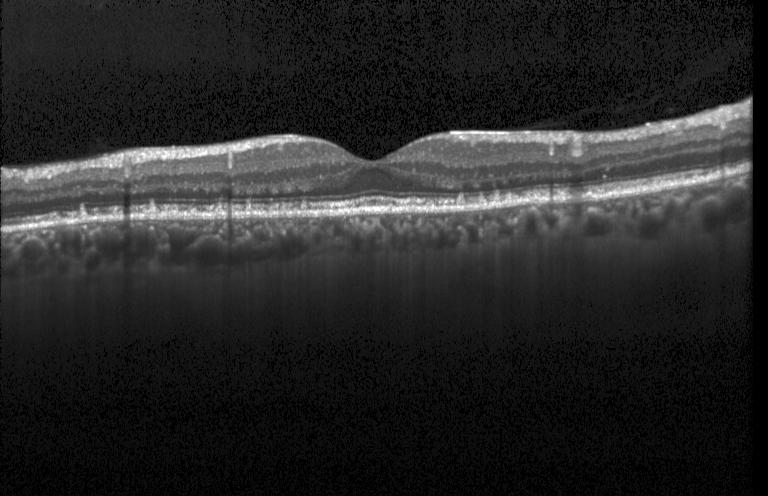
Spectral-domain optical coherence tomography, through the macula, instrument: Heidelberg Spectralis, retinal OCT cross-section.
Multiple drusen.